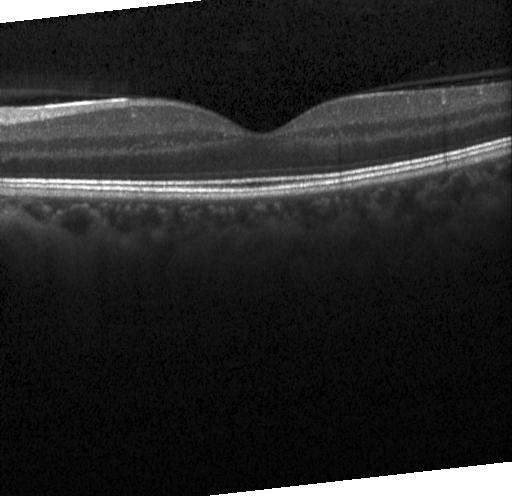 Spectral-domain optical coherence tomography; optical coherence tomography scan; Heidelberg Spectralis OCT system
OCT finding: no CNV, no DME, and no drusen.